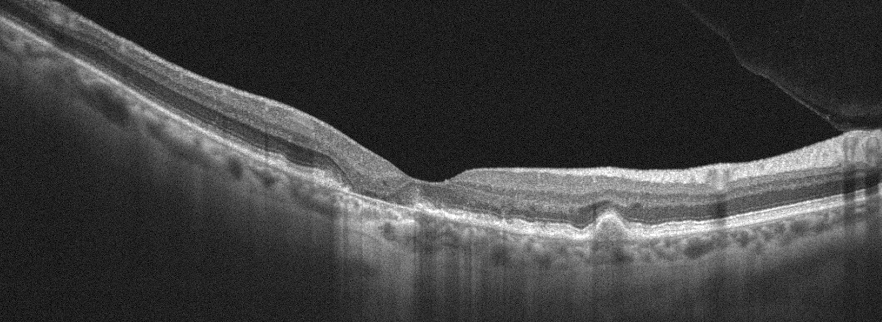 OCT B-scan. OS. Diagnosis: AMD.